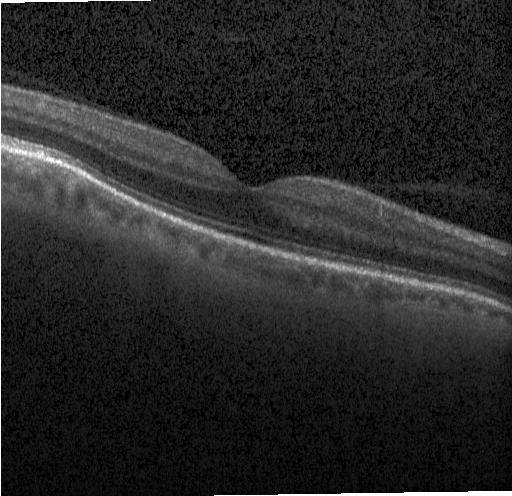
Retinal OCT B-scan · Heidelberg Spectralis OCT system · spectral-domain OCT · through the macula
Finding: neither choroidal neovascularization, diabetic macular edema, nor drusen.